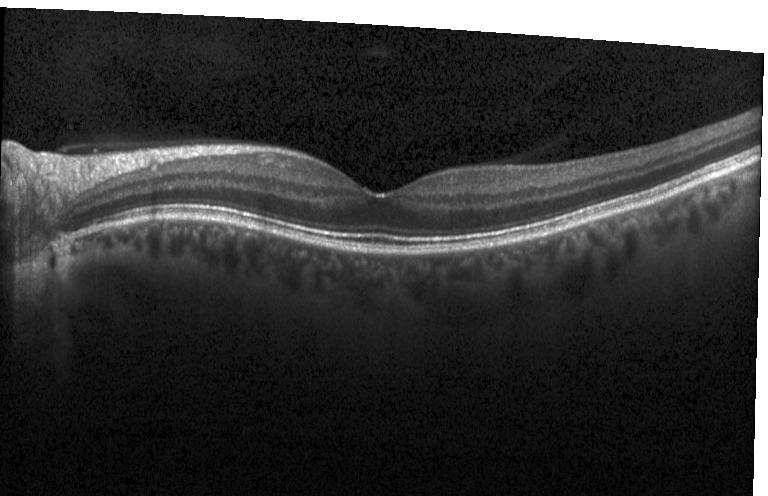

Impression: no choroidal neovascularization, diabetic macular edema, or drusen.